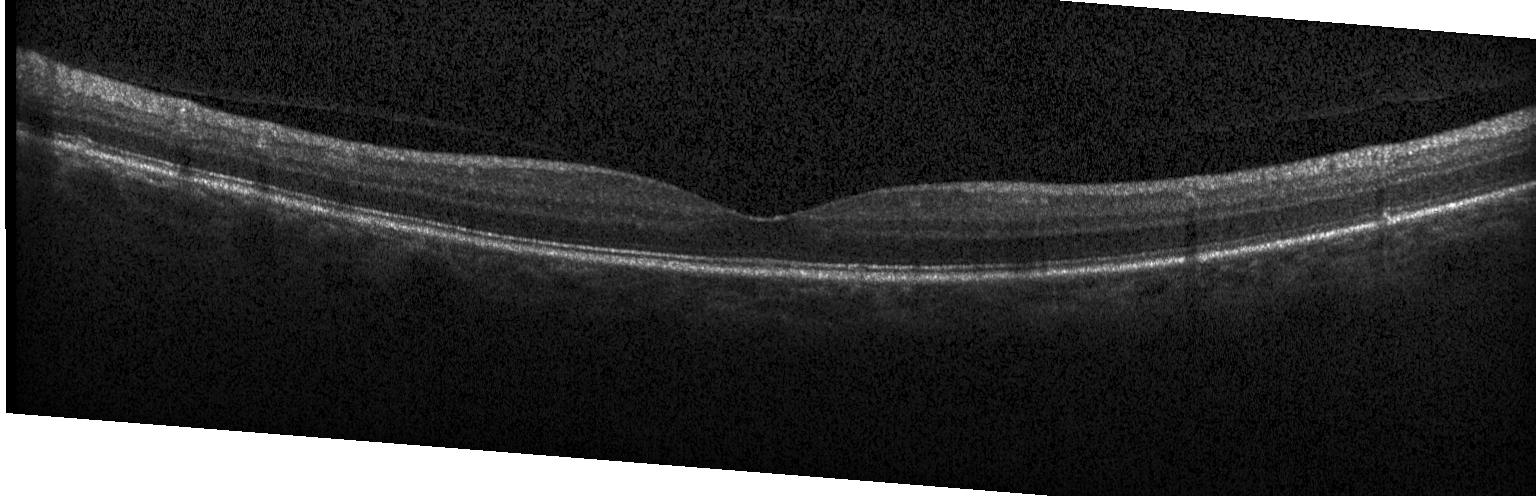
Optical coherence tomography B-scan, spectral-domain optical coherence tomography, fovea-centered, Heidelberg Spectralis.
Assessment: no CNV, no DME, and no drusen.